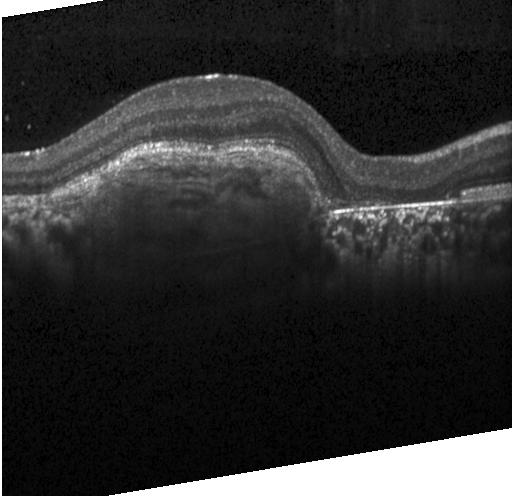
OCT B-scan showing a choroidal neovascular membrane.